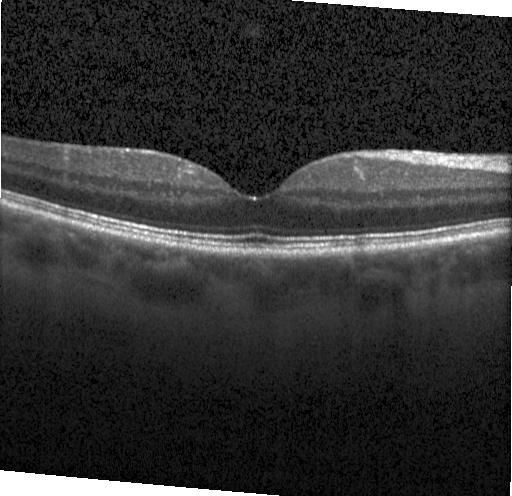
Optical coherence tomography B-scan, spectral-domain optical coherence tomography, instrument: Heidelberg Spectralis, horizontal scan through the fovea. Impression: no evidence of CNV, DME, or drusen.